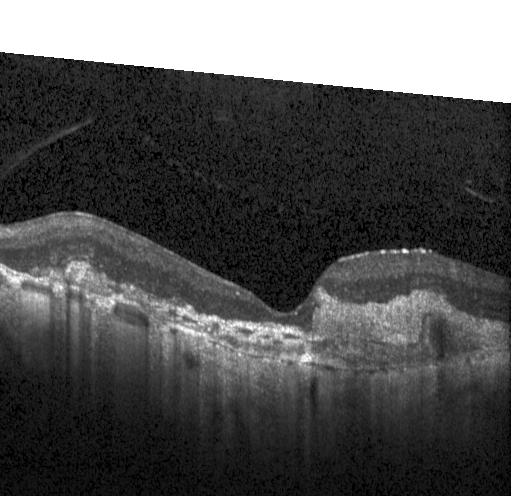

Diagnosis: a choroidal neovascular membrane.